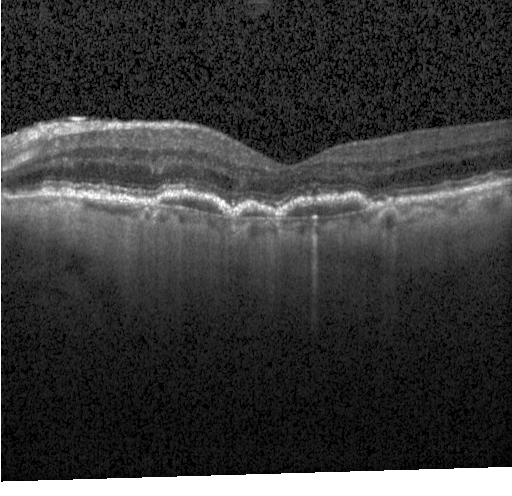

Retinal OCT cross-section — A choroidal neovascular membrane.